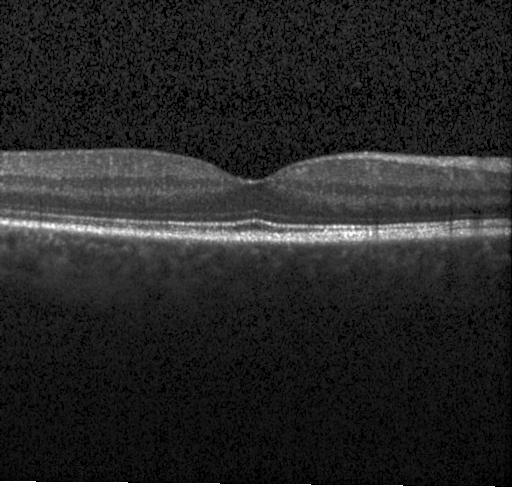 Retinal OCT cross-section. Instrument: Heidelberg Spectralis. Through the macula. Spectral-domain OCT.
Diagnosis: no CNV, DME, or drusen.